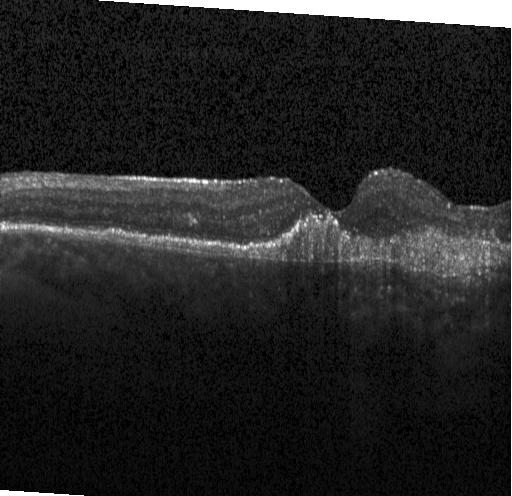
Retinal OCT cross-section showing a choroidal neovascular membrane.